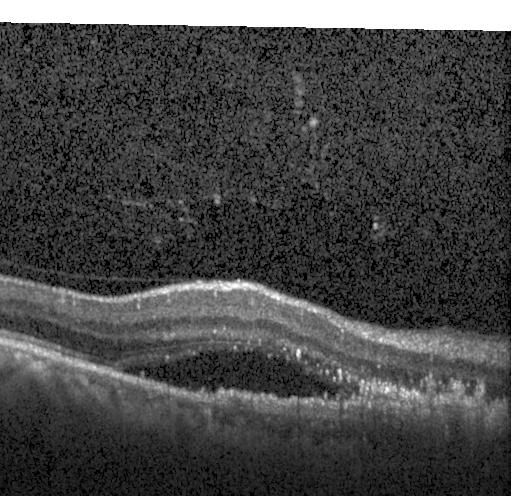

Macular scan, OCT line scan, acquired on a Heidelberg Spectralis, SD-OCT
This B-scan demonstrates choroidal neovascularization.